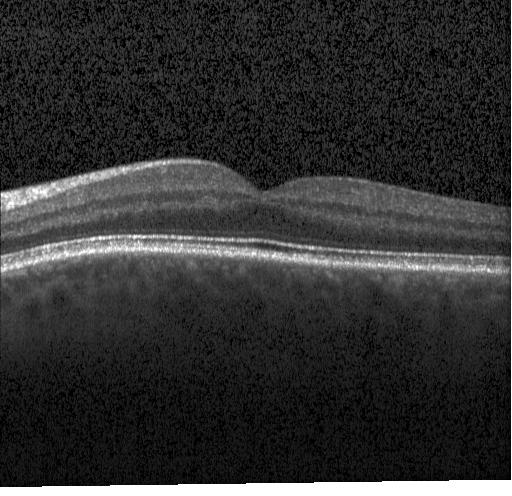

Impression: neither choroidal neovascularization, diabetic macular edema, nor drusen.